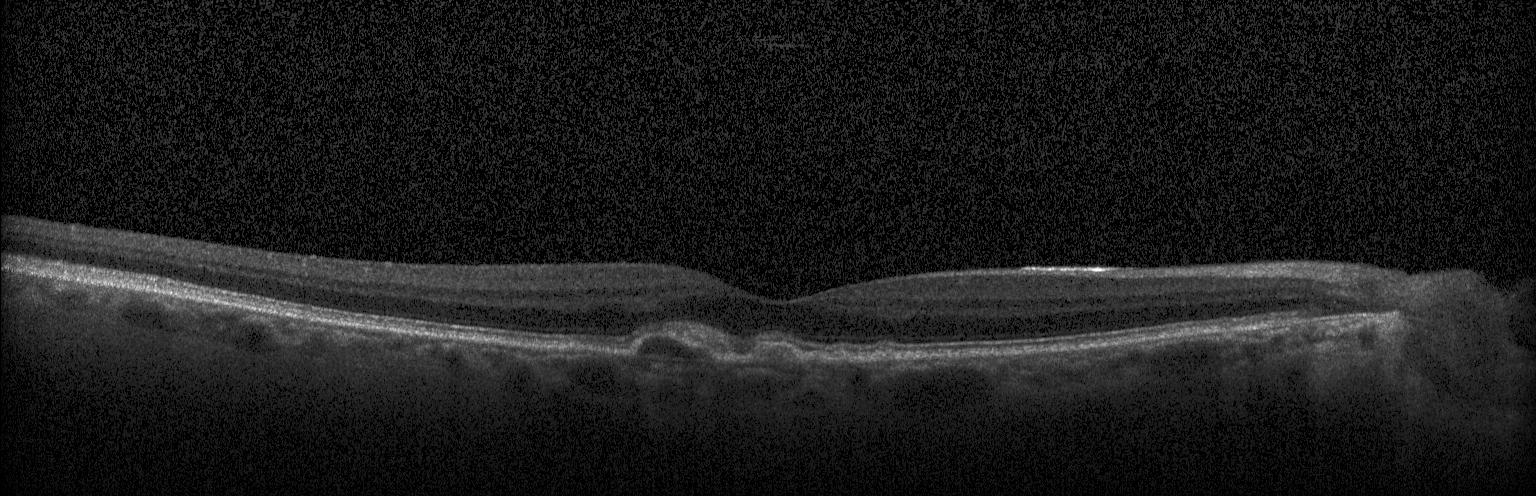 OCT line scan. Spectral-domain optical coherence tomography. Through the macula — Impression: choroidal neovascularization.